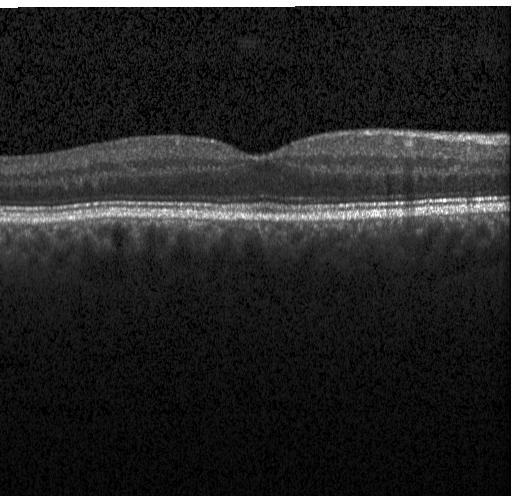 Through the macula · optical coherence tomography B-scan — The scan shows no CNV, DME, or drusen.